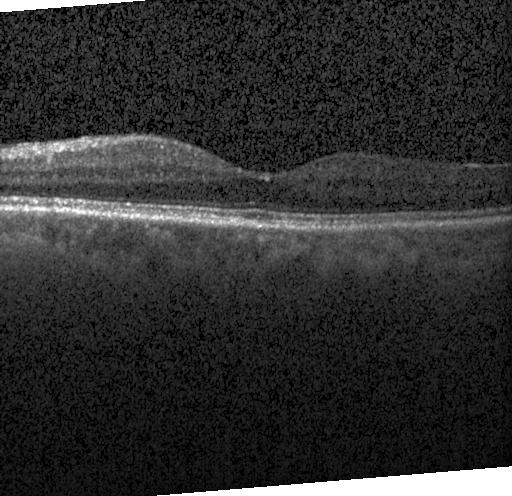
SD-OCT; retinal OCT cross-section; fovea-centered.
Impression: no choroidal neovascularization, diabetic macular edema, or drusen.